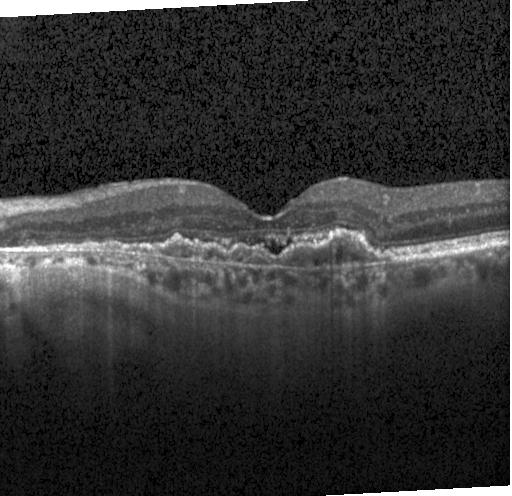

OCT line scan, fovea-centered. Macular OCT: a choroidal neovascular membrane.